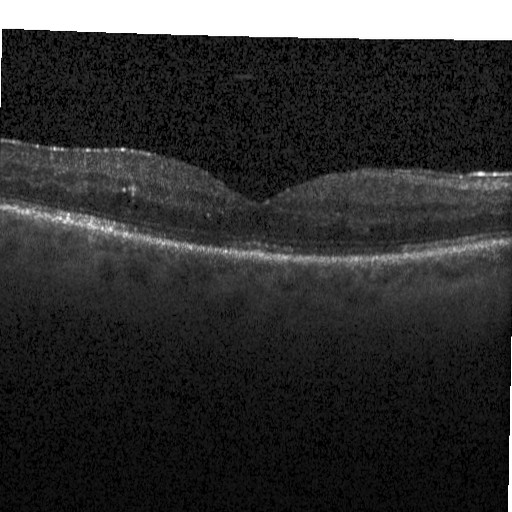
Centered on the fovea. Heidelberg Spectralis OCT system. Retinal OCT B-scan. Spectral-domain OCT — Assessment: DME.